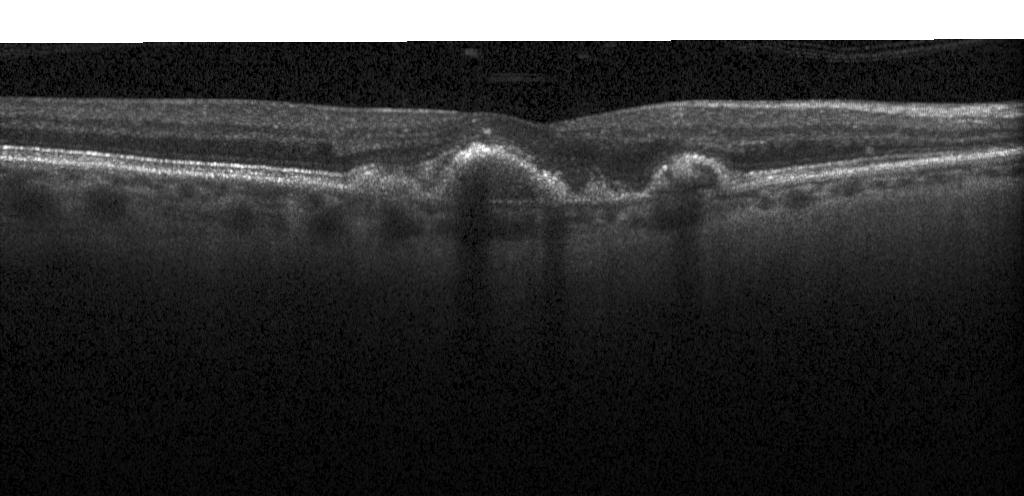

SD-OCT · retinal OCT cross-section.
Impression: a choroidal neovascular membrane.